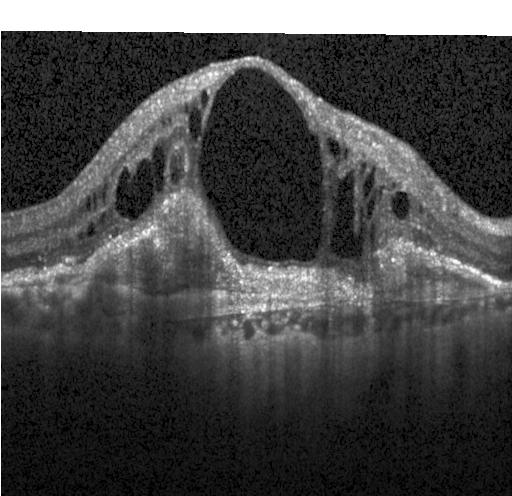
Diagnosis: choroidal neovascularization.